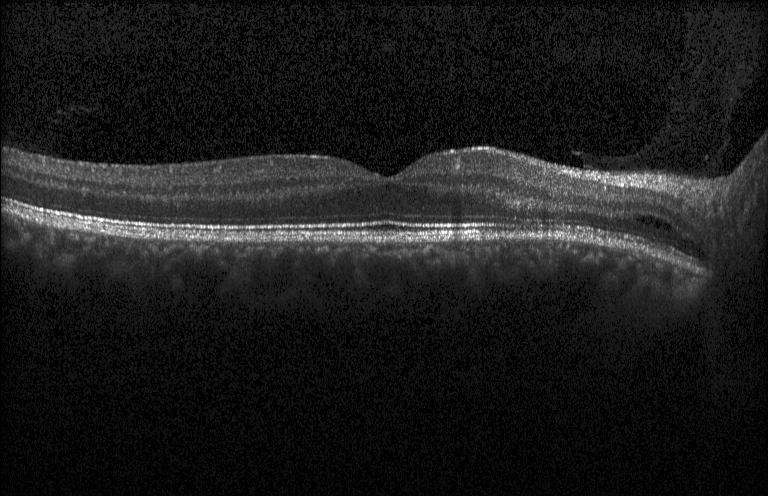
OCT B-scan
Diagnosis: diabetic macular edema (DME).